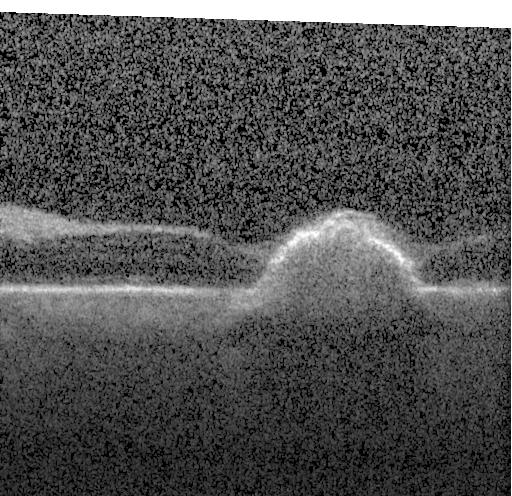 OCT line scan — Diagnosis: a choroidal neovascular membrane.